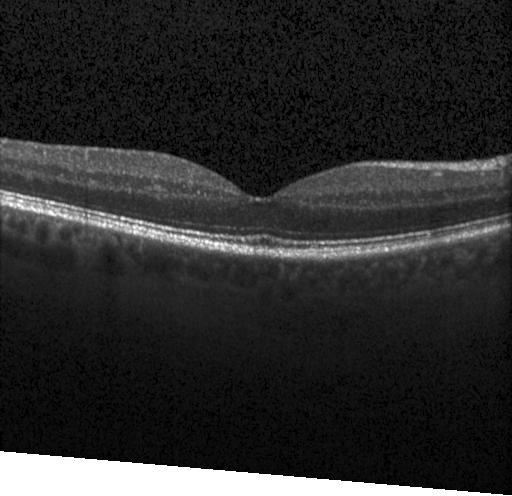

Macular OCT demonstrating no choroidal neovascularization, no diabetic macular edema, and no drusen.